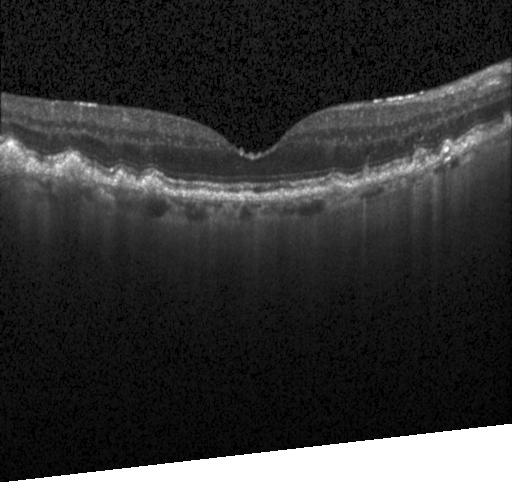
OCT line scan · horizontal scan through the fovea · Heidelberg Spectralis OCT system.
Finding: drusen.